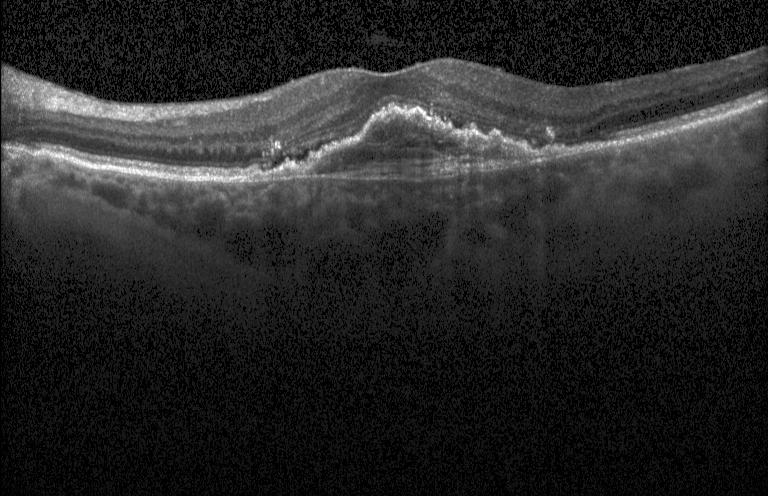

Horizontal scan through the fovea; SD-OCT; acquired on a Heidelberg Spectralis; OCT line scan — Finding: CNV.